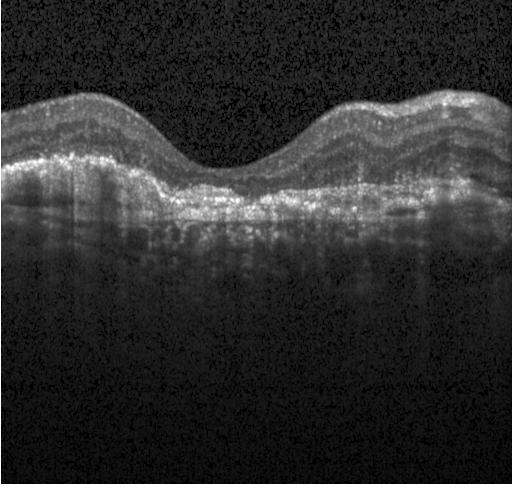
Spectral-domain OCT, OCT line scan — Finding: choroidal neovascularization.